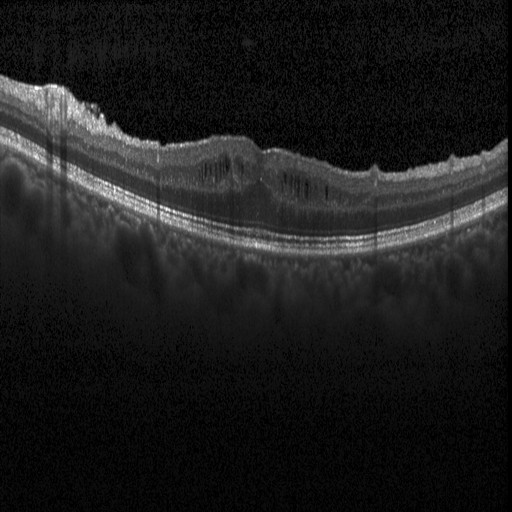
OCT line scan; spectral-domain optical coherence tomography — Macular OCT: diabetic macular edema (DME).